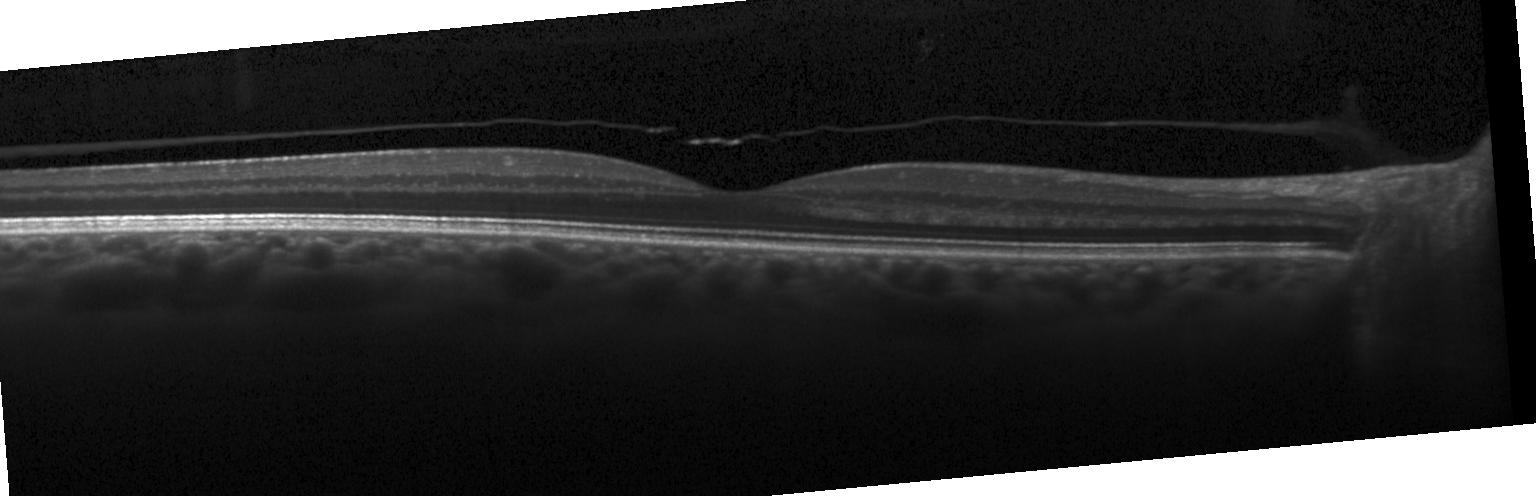
Centered on the fovea; retinal OCT B-scan; Heidelberg Spectralis; SD-OCT — Diagnosis: no evidence of CNV, DME, or drusen.